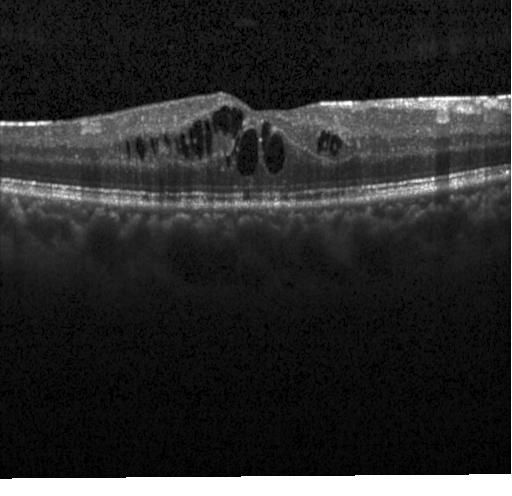

Horizontal scan through the fovea; OCT line scan; SD-OCT.
OCT finding: diabetic macular edema.